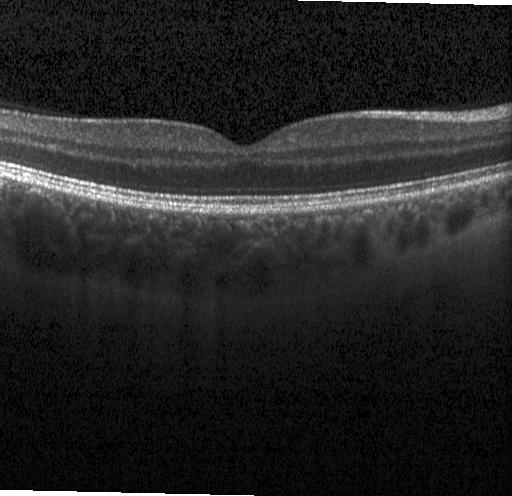 OCT B-scan · spectral-domain OCT · centered on the fovea · Heidelberg Spectralis OCT system — Assessment: neither CNV, DME, nor drusen.